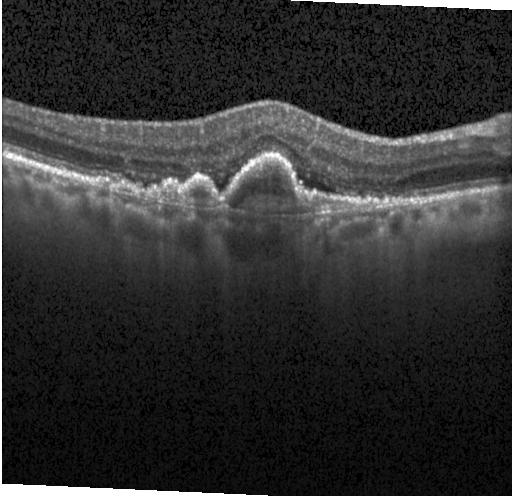

Diagnosis: a choroidal neovascular membrane.